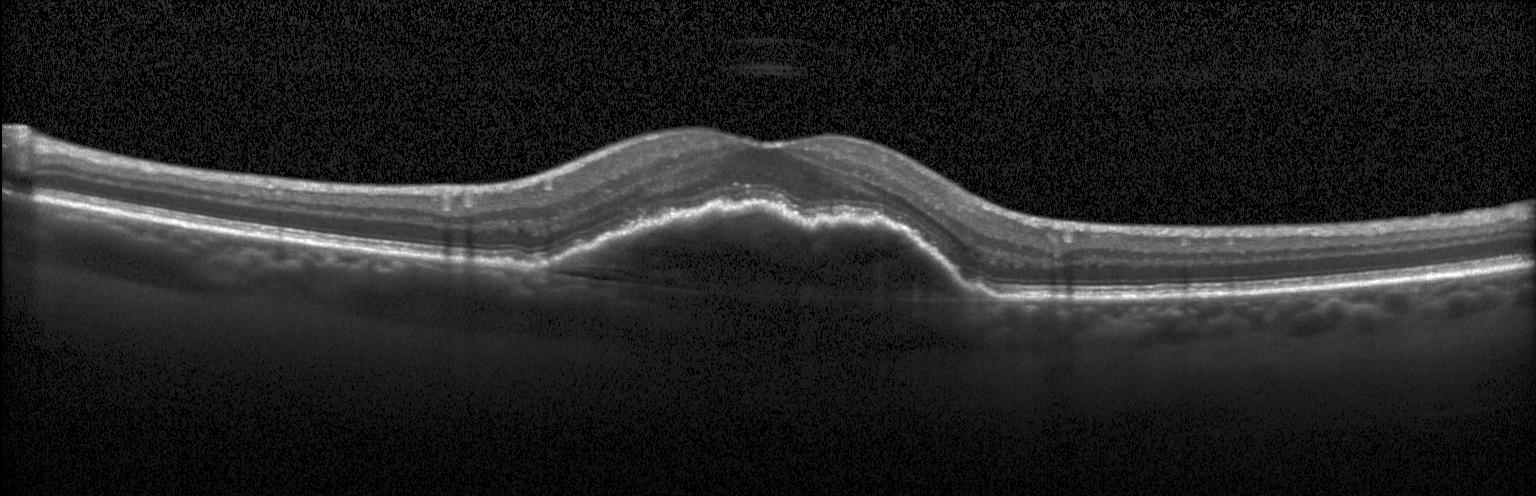

Spectral-domain optical coherence tomography · acquired on a Heidelberg Spectralis · optical coherence tomography scan.
Macular OCT: choroidal neovascularization (CNV).